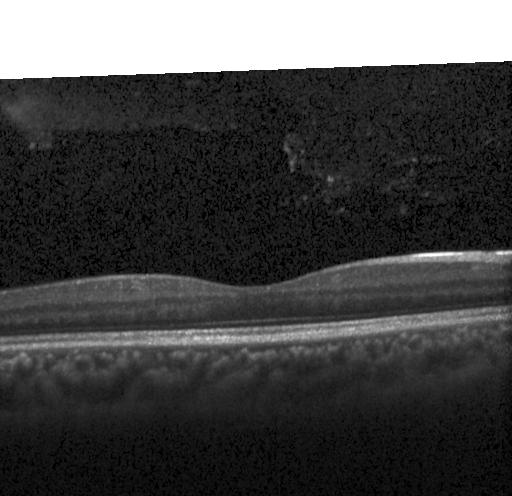 Optical coherence tomography B-scan — OCT finding: no choroidal neovascularization, no diabetic macular edema, and no drusen.